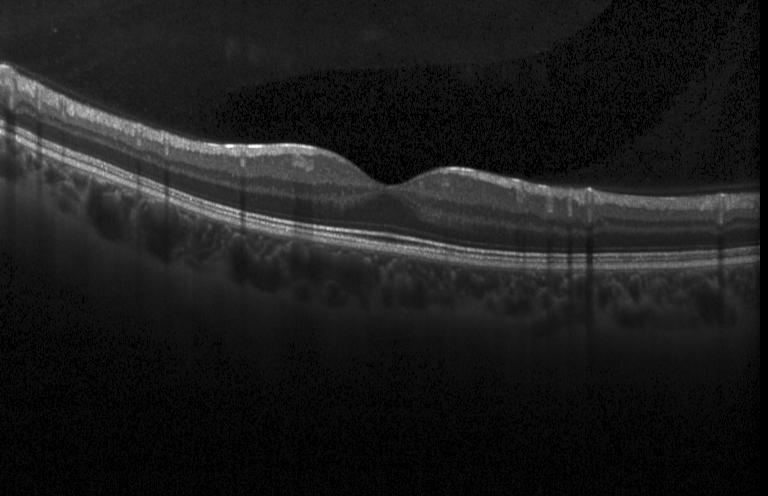 Instrument: Heidelberg Spectralis · SD-OCT · retinal OCT B-scan — Assessment: no CNV, no DME, and no drusen.